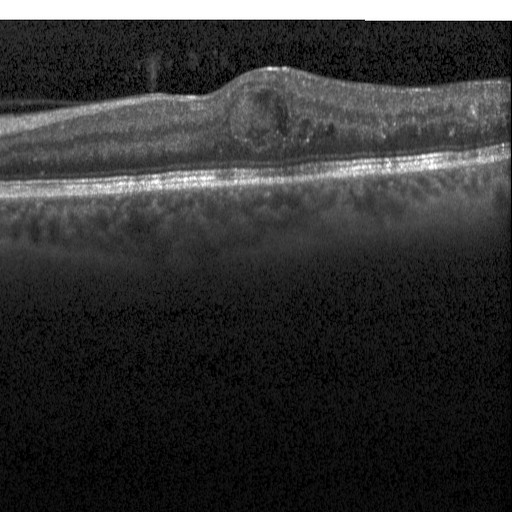 Retinal OCT cross-section; spectral-domain optical coherence tomography
Impression: diabetic macular edema (DME).